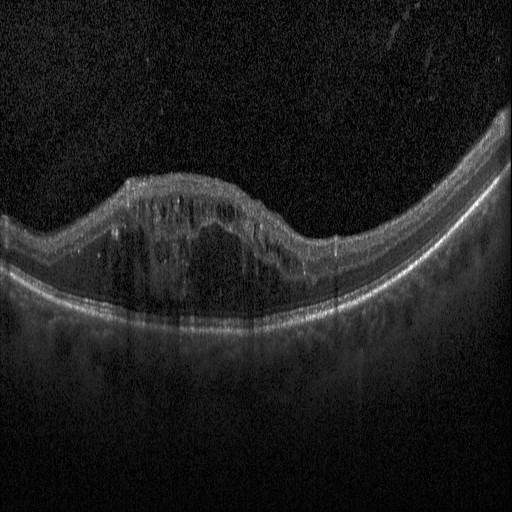
Spectral-domain optical coherence tomography · retinal OCT B-scan · horizontal scan through the fovea.
Diagnosis: diabetic macular edema (DME).